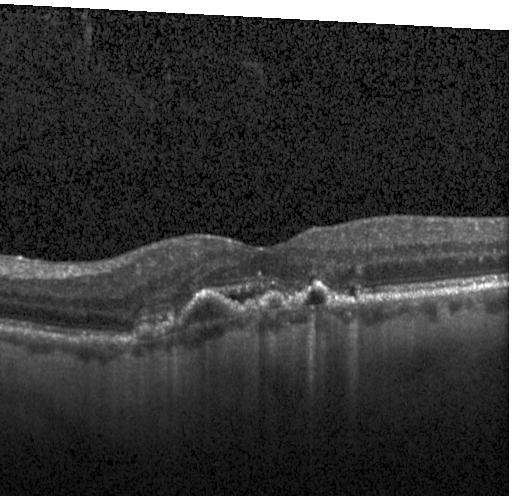
Assessment: a choroidal neovascular membrane.